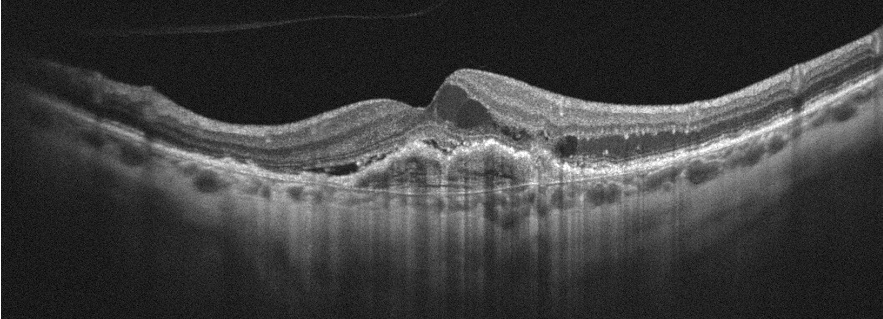 Optical coherence tomography B-scan — The scan shows age-related macular degeneration (AMD).